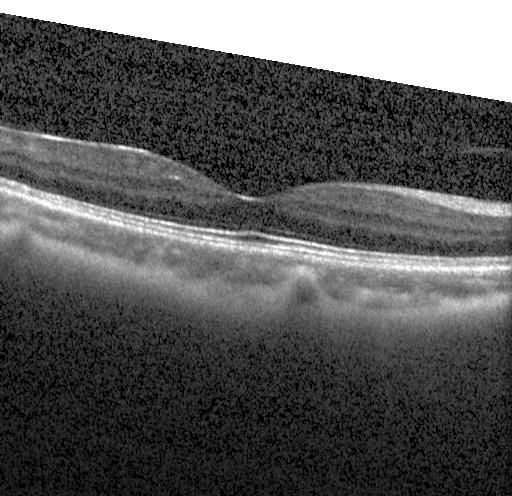 Optical coherence tomography B-scan. Spectral-domain OCT. Dx: neither choroidal neovascularization, diabetic macular edema, nor drusen.